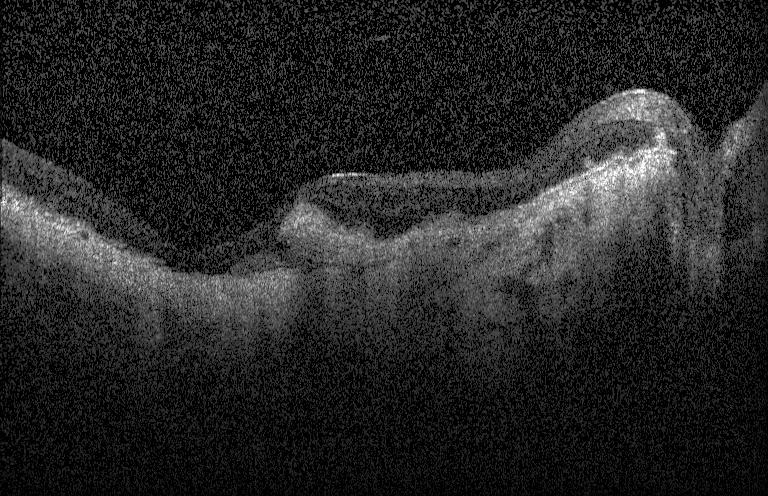
Acquired on a Heidelberg Spectralis, OCT line scan.
This B-scan demonstrates choroidal neovascularization.